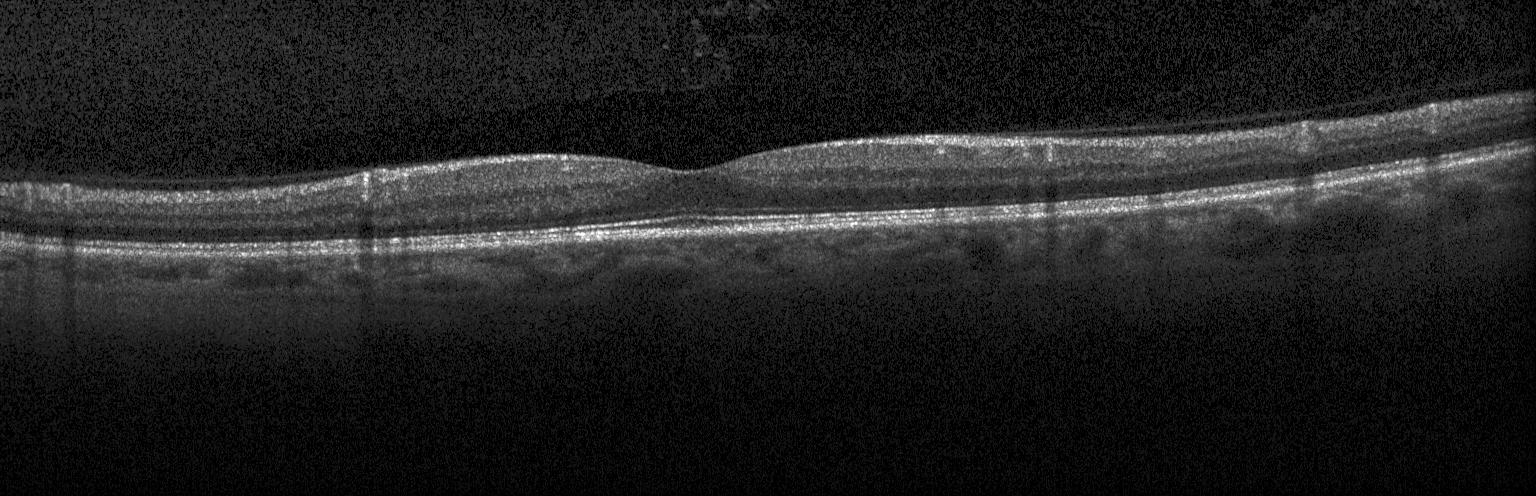 Through the macula. Acquired on a Heidelberg Spectralis. Spectral-domain OCT. Optical coherence tomography scan.
Assessment: neither choroidal neovascularization, diabetic macular edema, nor drusen.